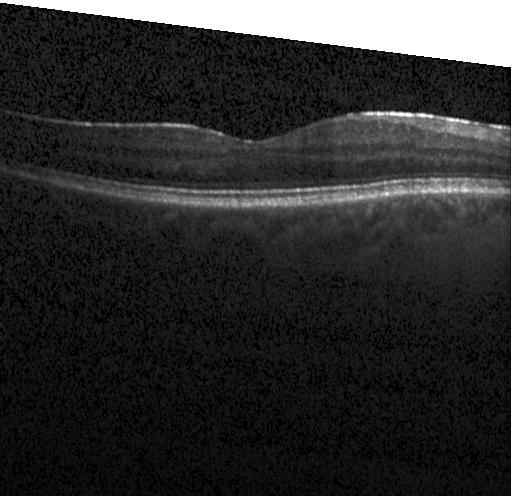

Heidelberg Spectralis; centered on the fovea; retinal OCT cross-section; SD-OCT. Finding: no evidence of choroidal neovascularization, diabetic macular edema, or drusen.